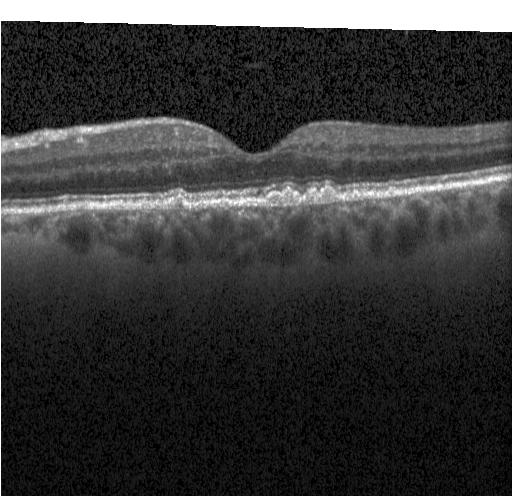
OCT B-scan showing multiple drusen.